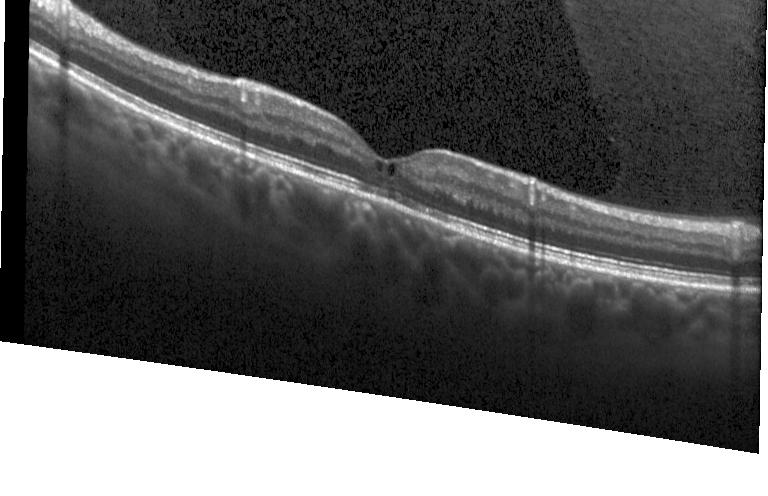 OCT line scan.
Dx: diabetic macular edema.